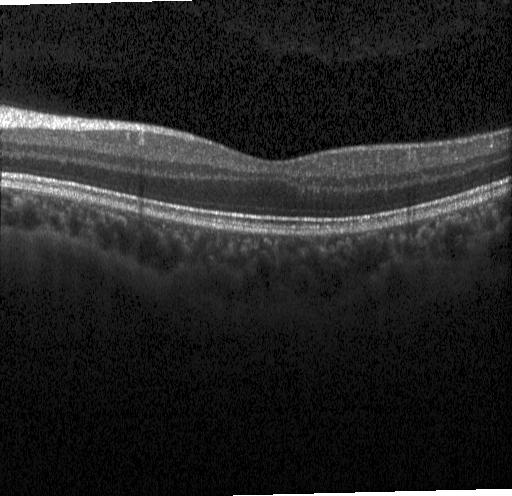 Heidelberg Spectralis, optical coherence tomography B-scan — The scan shows no CNV, no DME, and no drusen.